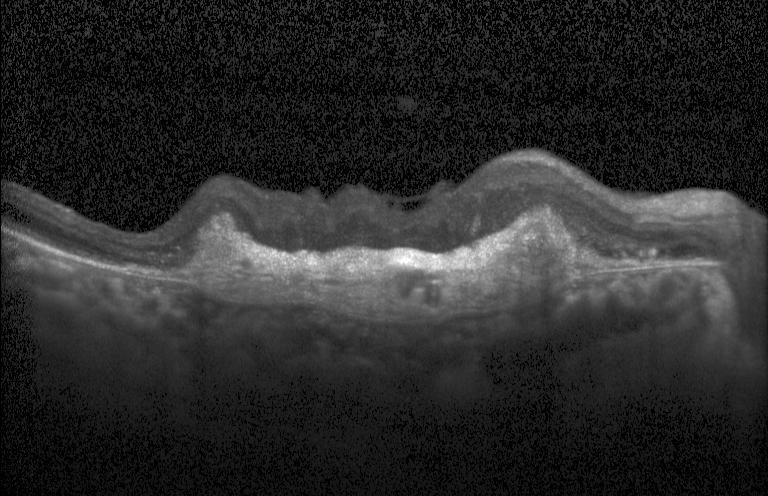 SD-OCT, Heidelberg Spectralis OCT system, horizontal scan through the fovea, retinal OCT cross-section
Diagnosis: CNV.